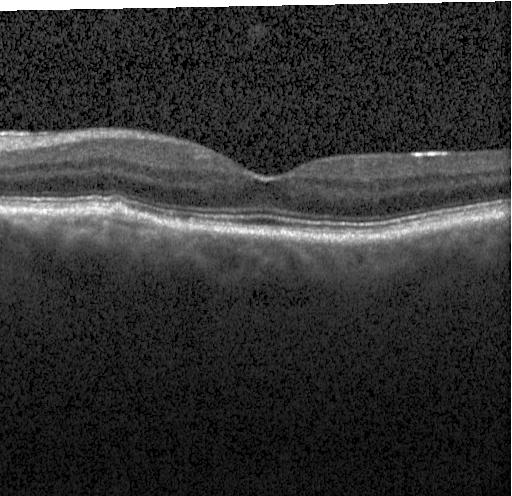

This B-scan demonstrates multiple drusen.